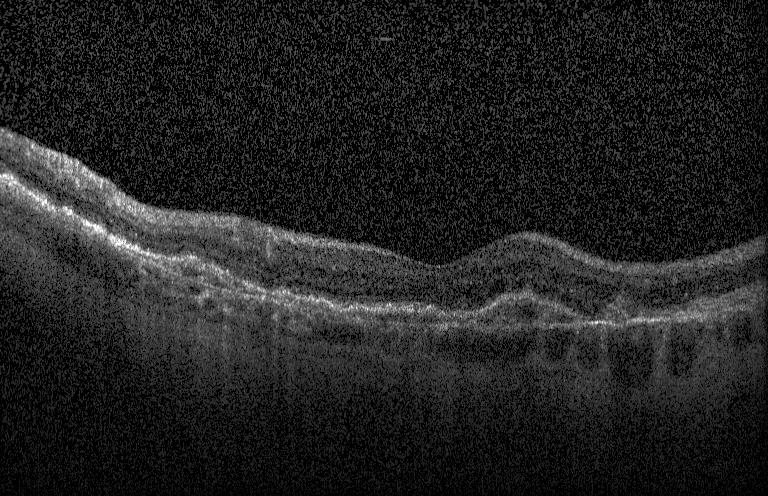
Acquired on a Heidelberg Spectralis; retinal OCT B-scan; macular scan — Assessment: a choroidal neovascular membrane.